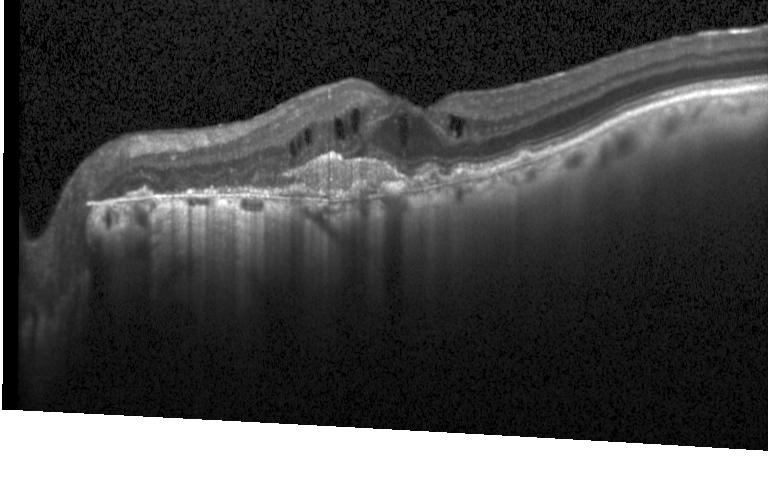
Fovea-centered; Heidelberg Spectralis; SD-OCT; retinal OCT B-scan.
Finding: choroidal neovascularization (CNV).